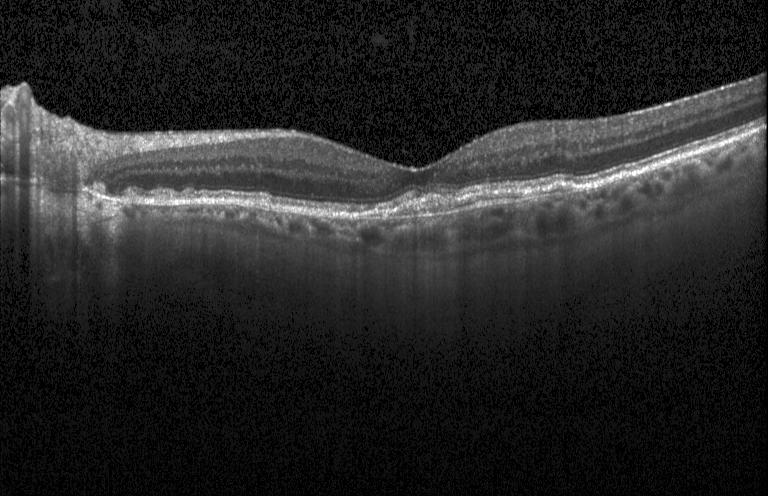
Retinal OCT cross-section showing a choroidal neovascular membrane.